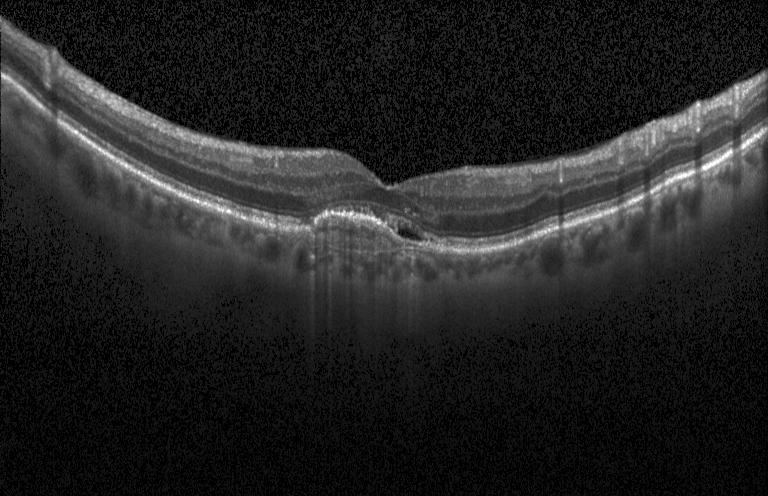 OCT line scan; spectral-domain optical coherence tomography; acquired on a Heidelberg Spectralis — Impression: a choroidal neovascular membrane.